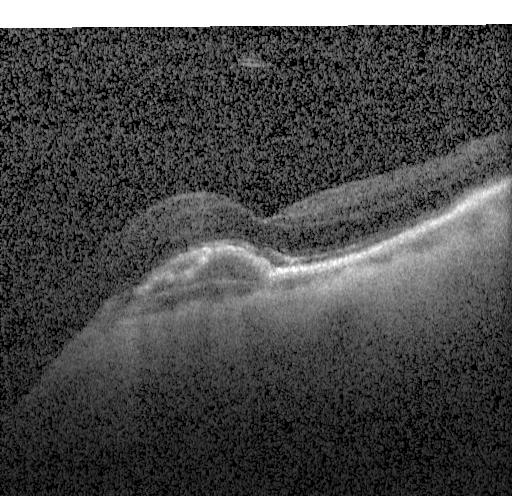
Heidelberg Spectralis OCT system. Optical coherence tomography scan
OCT finding: choroidal neovascularization.